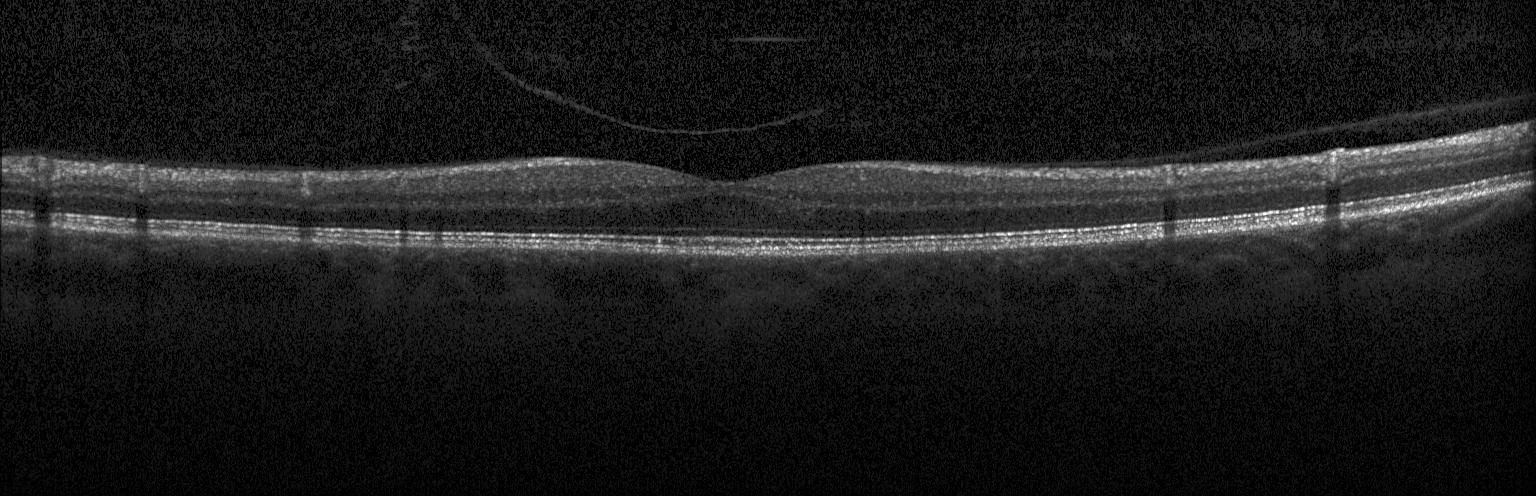 OCT scan showing neither choroidal neovascularization, diabetic macular edema, nor drusen.